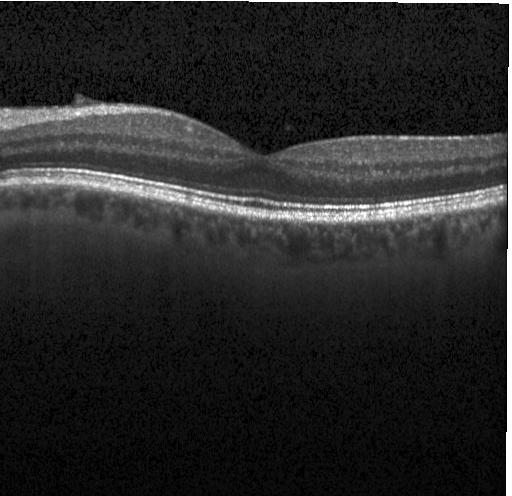

Macular OCT: no CNV, DME, or drusen.